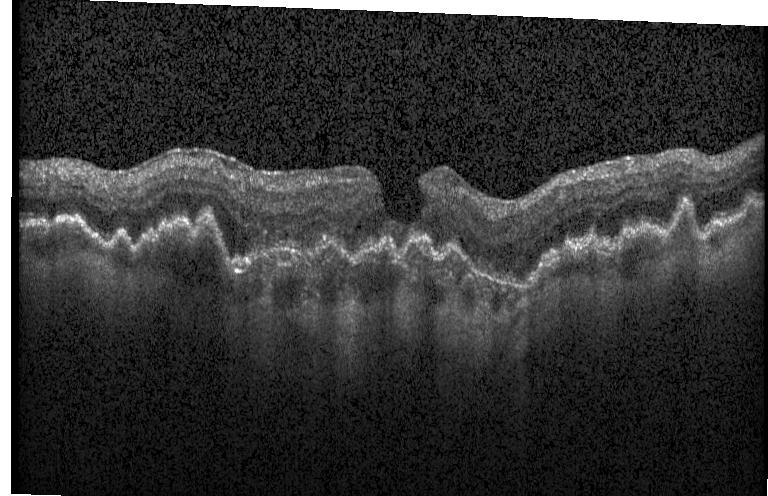
Diagnosis: choroidal neovascularization (CNV).